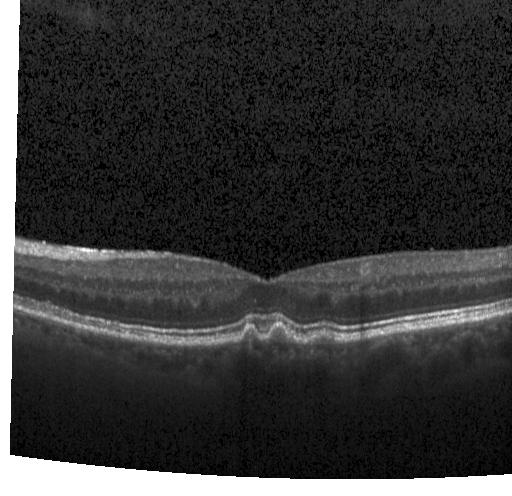
OCT B-scan; through the macula — Diagnosis: drusen.